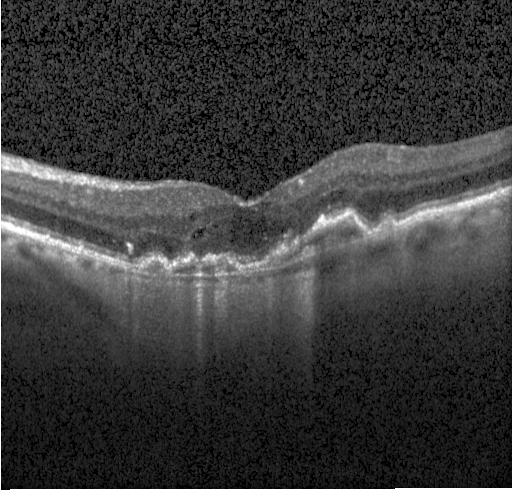 Retinal OCT B-scan, Heidelberg Spectralis, macular scan, SD-OCT — Finding: choroidal neovascularization.